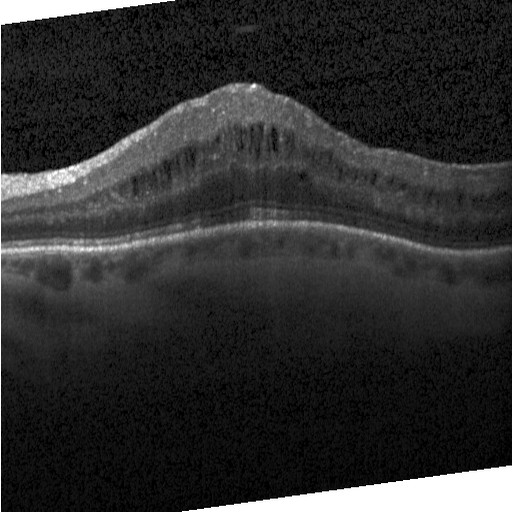 Acquired on a Heidelberg Spectralis, optical coherence tomography scan — The scan shows DME.